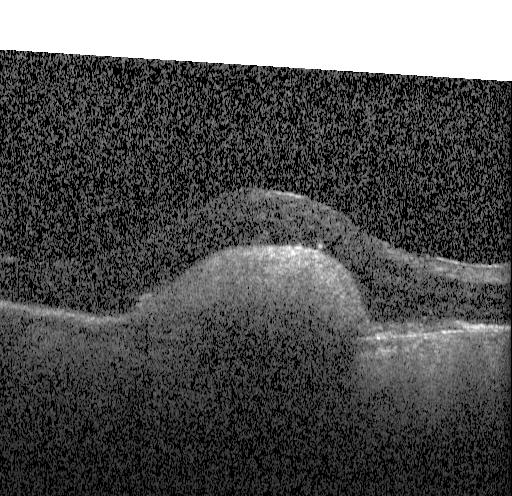

Assessment: choroidal neovascularization (CNV).